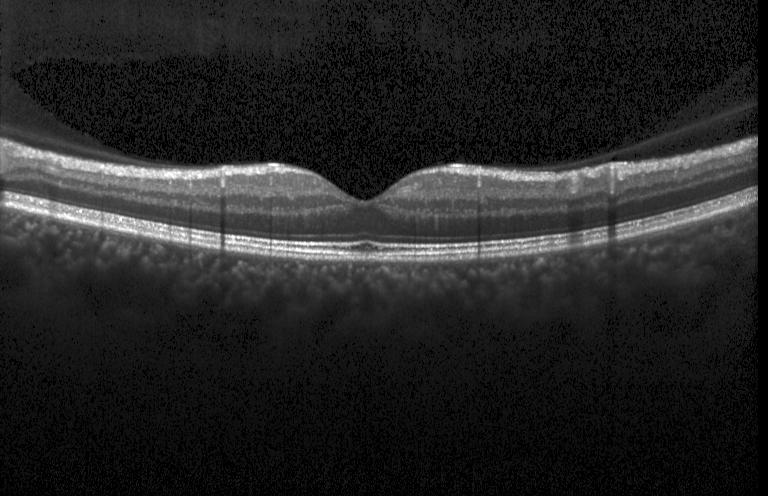 The scan shows no evidence of CNV, DME, or drusen.